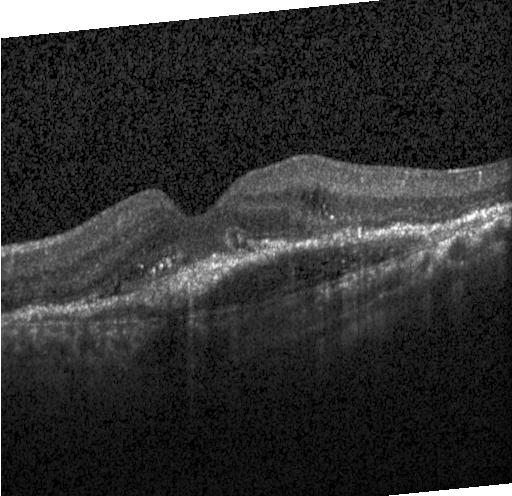

Optical coherence tomography B-scan. Diagnosis: choroidal neovascularization.